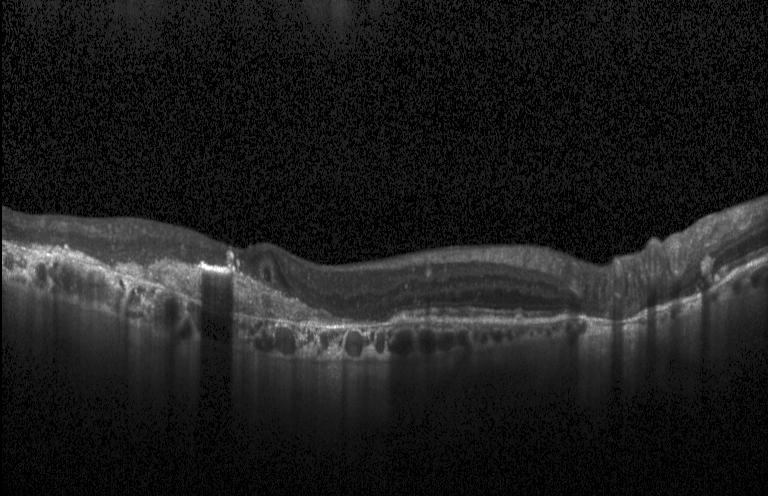

Spectral-domain OCT B-scan: a choroidal neovascular membrane.